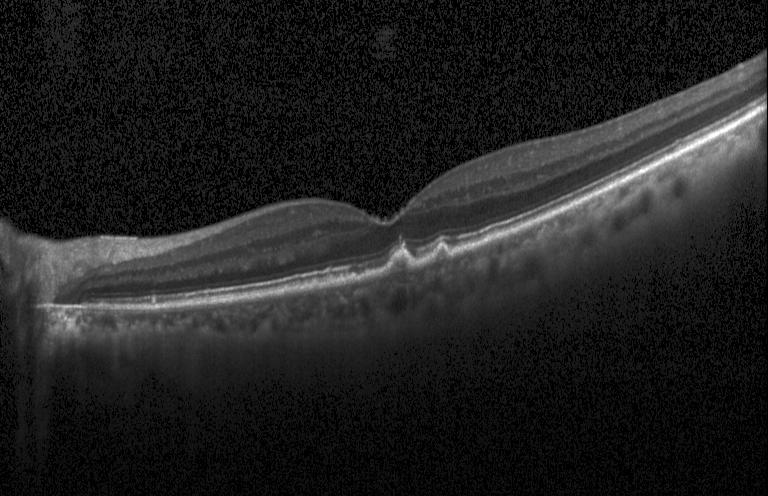
Assessment: drusen.